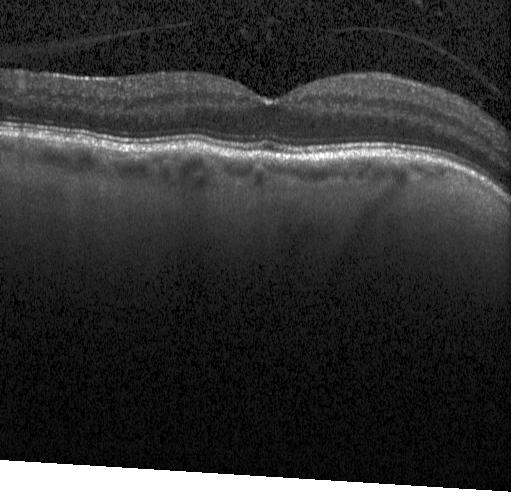

The scan shows no CNV, no DME, and no drusen.